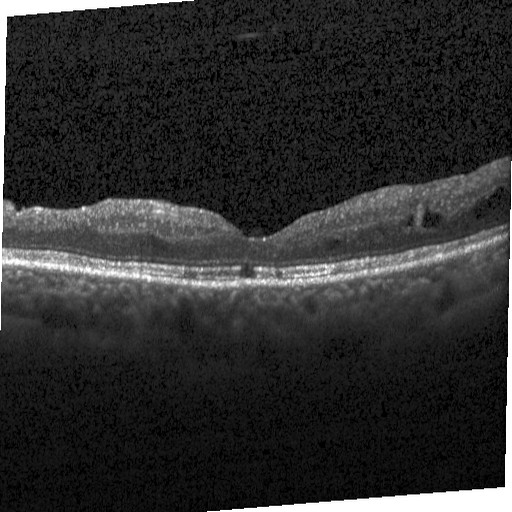 OCT B-scan; spectral-domain OCT; Heidelberg Spectralis.
Dx: diabetic macular edema (DME).